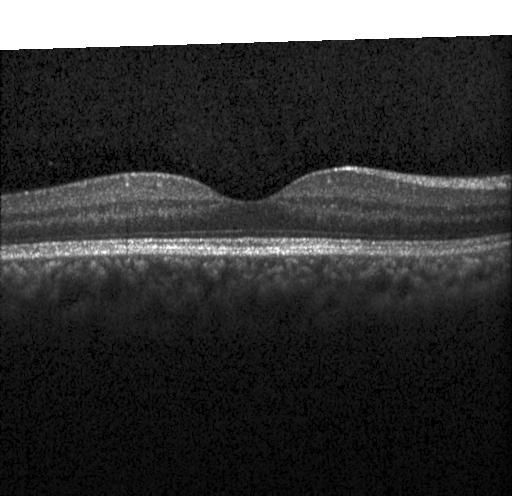

This B-scan demonstrates no evidence of choroidal neovascularization, diabetic macular edema, or drusen.